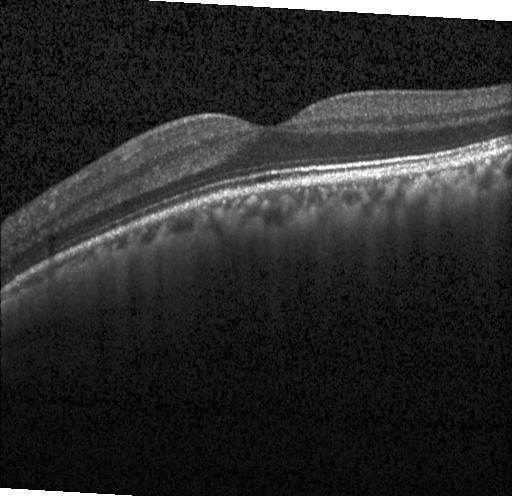 Finding: neither CNV, DME, nor drusen.